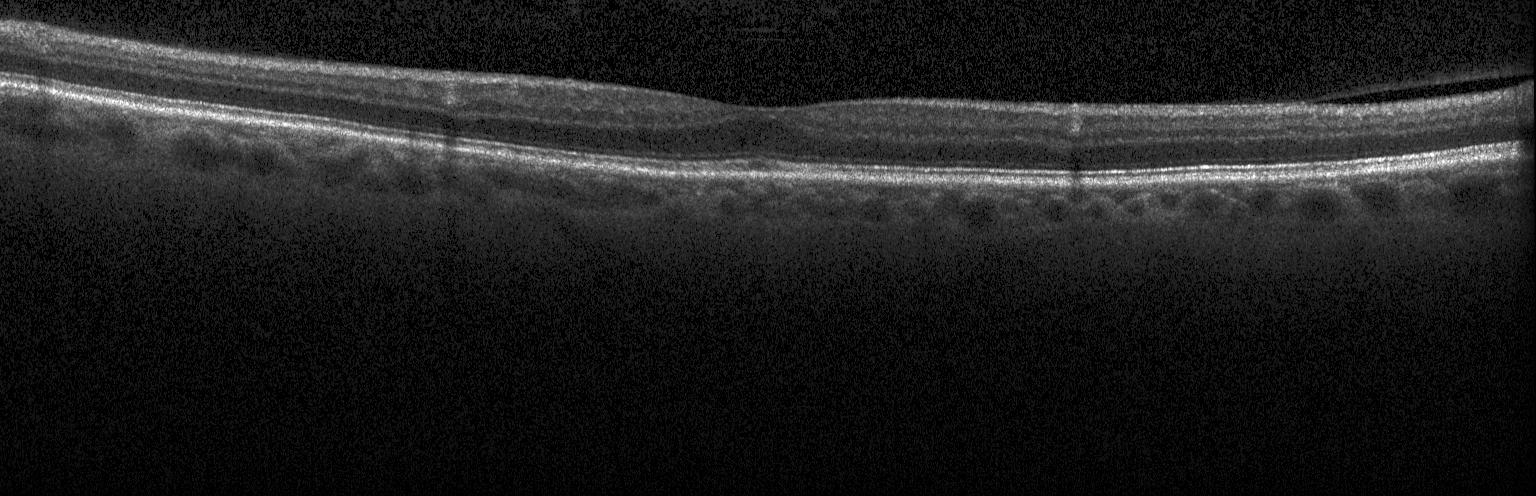
This B-scan demonstrates no choroidal neovascularization, diabetic macular edema, or drusen.